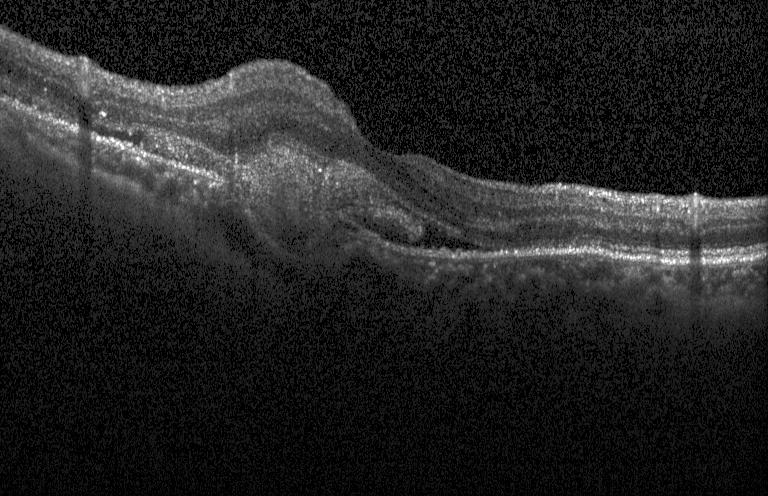
Optical coherence tomography B-scan
Choroidal neovascularization.